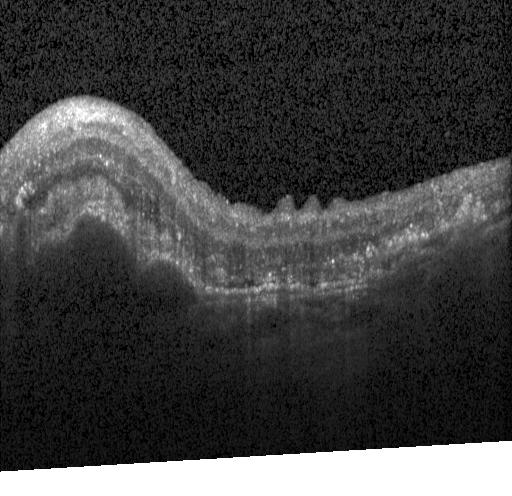
Retinal OCT B-scan. Heidelberg Spectralis OCT system. Macular scan — Assessment: CNV.